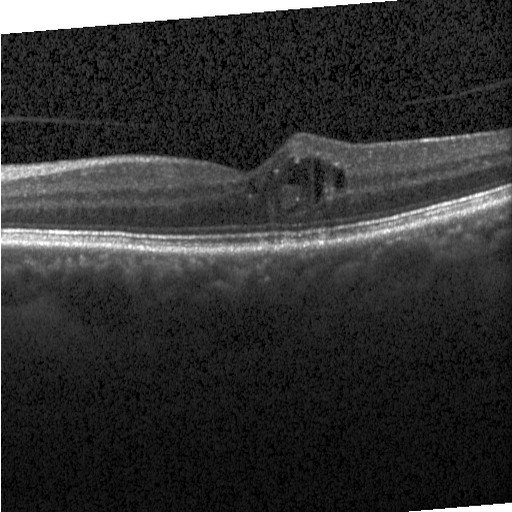 OCT line scan
The scan shows diabetic macular edema.